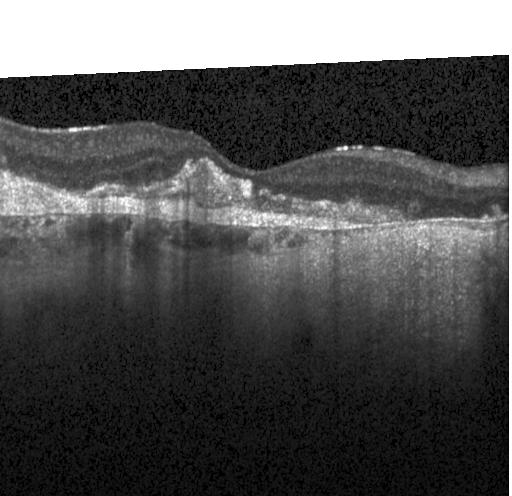
Optical coherence tomography scan
OCT finding: choroidal neovascularization (CNV).